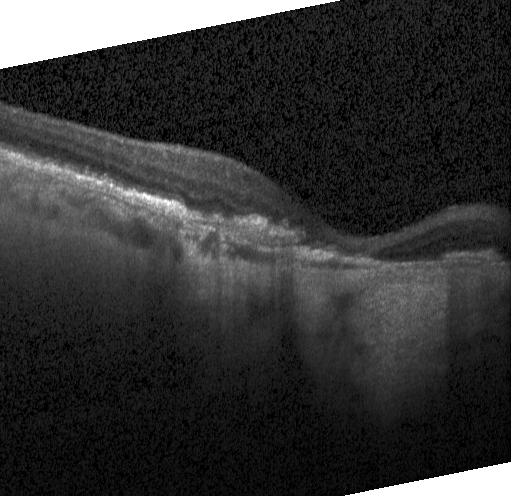 Spectral-domain OCT · retinal OCT B-scan
The scan shows choroidal neovascularization.